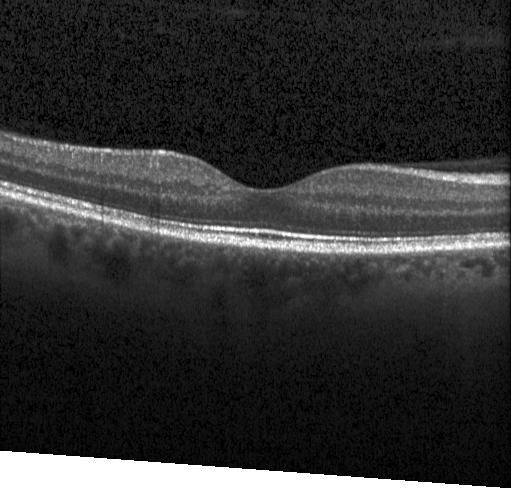
Heidelberg Spectralis OCT system. Horizontal scan through the fovea. SD-OCT. OCT B-scan
Impression: no choroidal neovascularization, diabetic macular edema, or drusen.